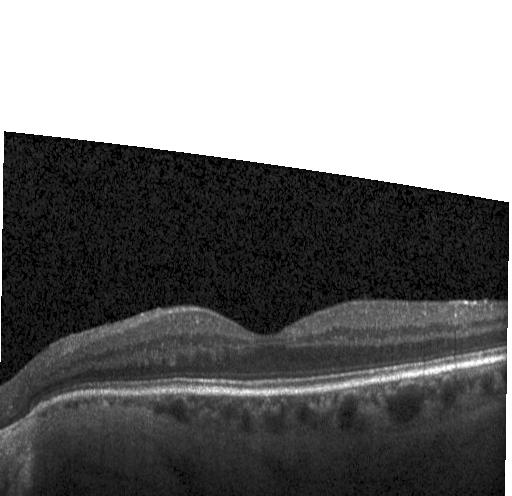

OCT finding: no choroidal neovascularization, diabetic macular edema, or drusen.